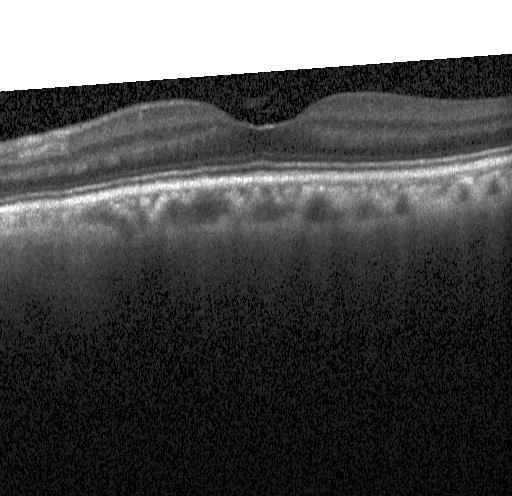 Retinal OCT cross-section showing no CNV, DME, or drusen.